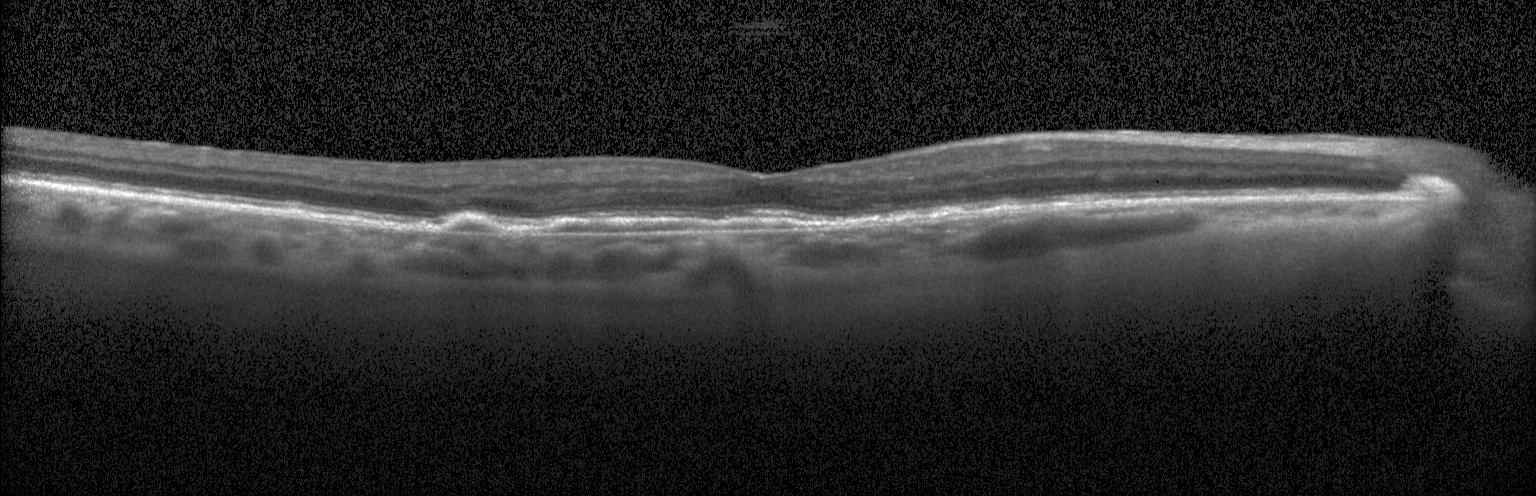

CNV.